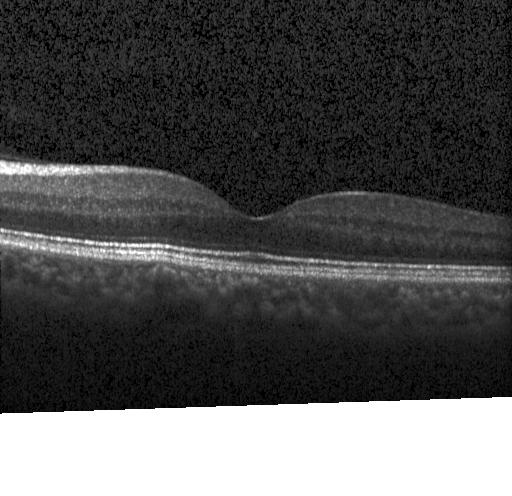
Optical coherence tomography scan. Finding: no evidence of CNV, DME, or drusen.